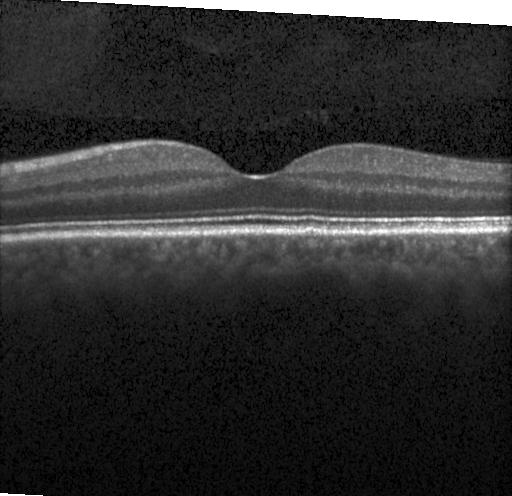
Assessment: no choroidal neovascularization, diabetic macular edema, or drusen.